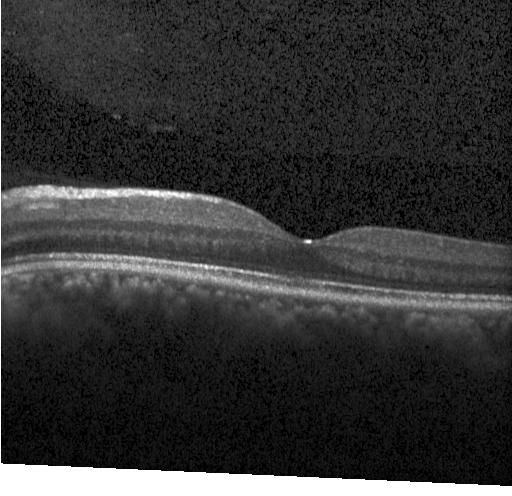
Retinal OCT cross-section showing no choroidal neovascularization, no diabetic macular edema, and no drusen.